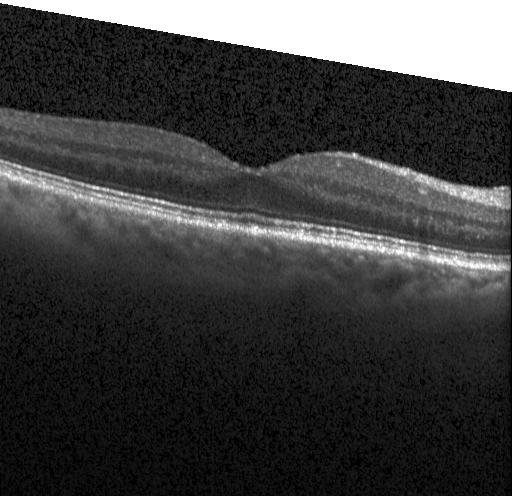
Retinal OCT B-scan
Finding: no choroidal neovascularization, diabetic macular edema, or drusen.